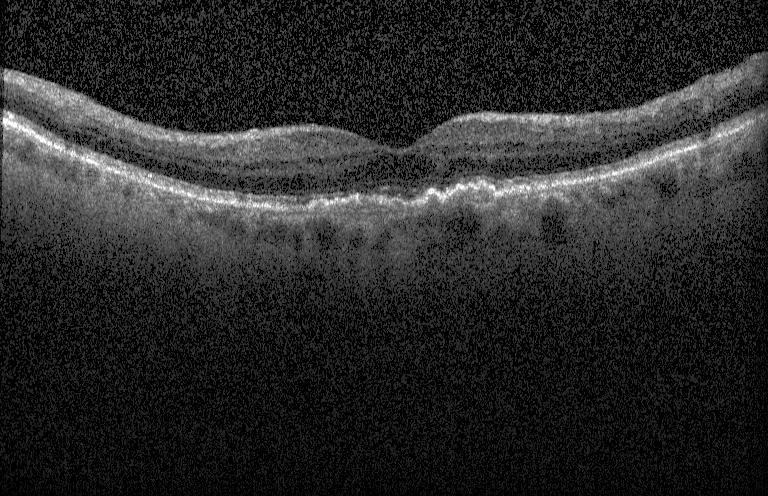
Optical coherence tomography B-scan. This B-scan demonstrates choroidal neovascularization.